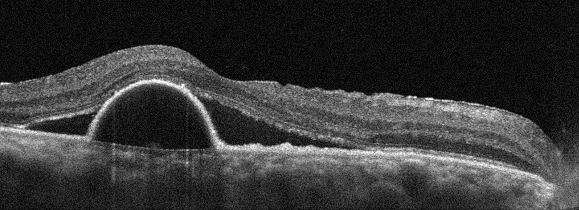 Right eye, retinal OCT B-scan
Finding: age-related macular degeneration.